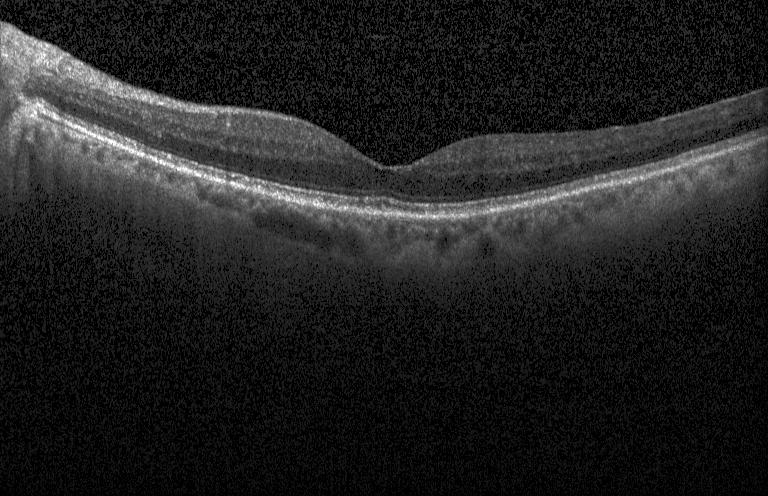 This B-scan demonstrates no choroidal neovascularization, no diabetic macular edema, and no drusen.